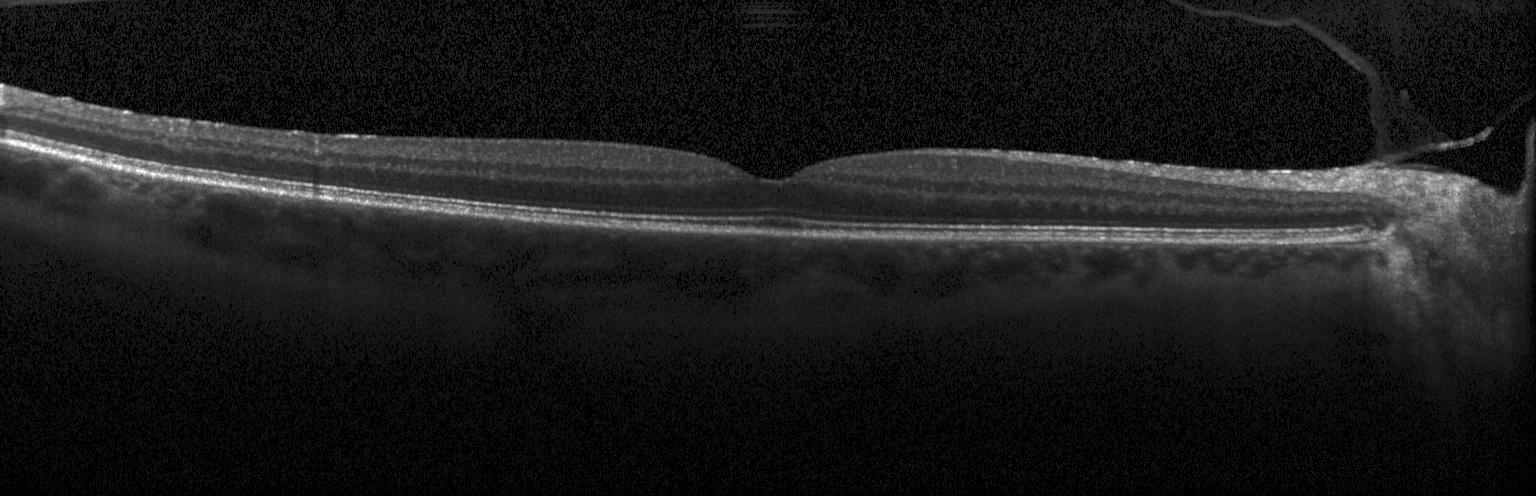 SD-OCT, optical coherence tomography B-scan, horizontal scan through the fovea. This B-scan demonstrates no choroidal neovascularization, diabetic macular edema, or drusen.